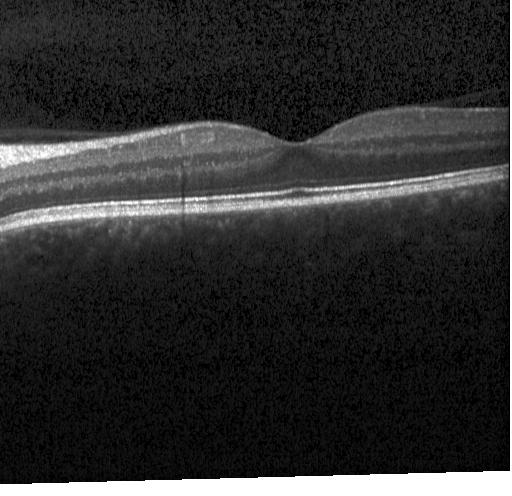

OCT line scan
Impression: no choroidal neovascularization, diabetic macular edema, or drusen.